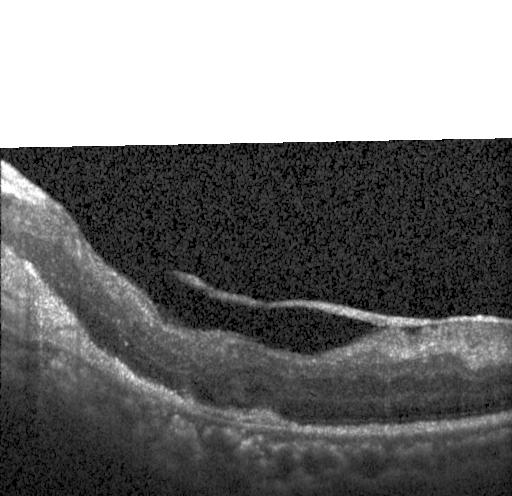
Heidelberg Spectralis. Retinal OCT B-scan.
Diagnosis: choroidal neovascularization.